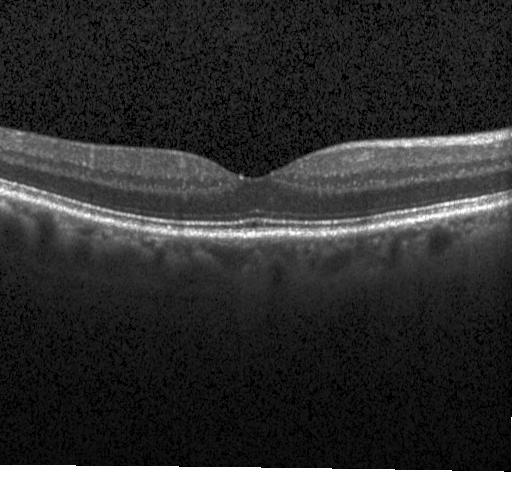

Optical coherence tomography scan · SD-OCT · acquired on a Heidelberg Spectralis. Finding: no CNV, DME, or drusen.